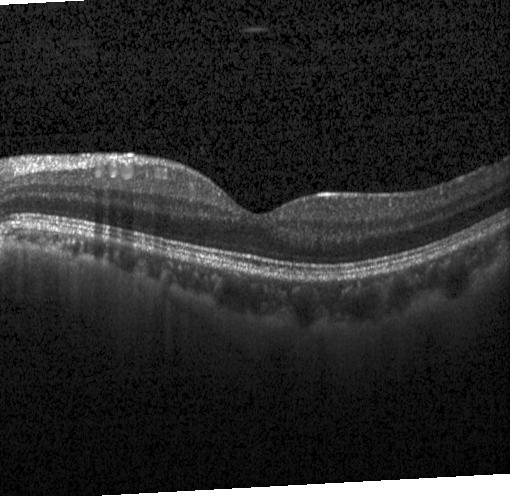

Dx: no evidence of choroidal neovascularization, diabetic macular edema, or drusen.